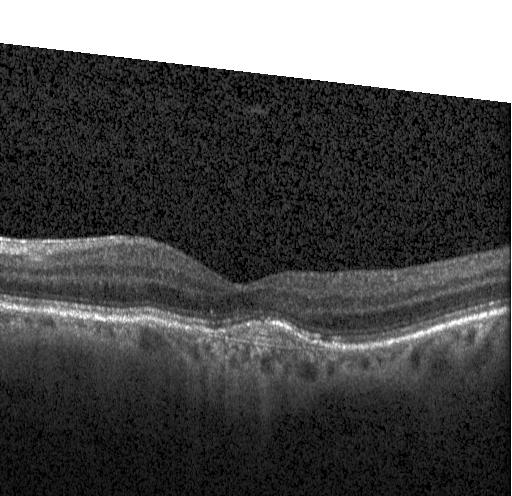 OCT line scan. Macular OCT: a choroidal neovascular membrane.